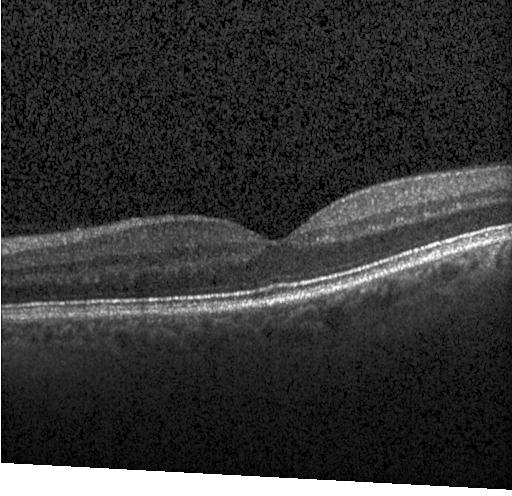 OCT line scan — The scan shows no evidence of CNV, DME, or drusen.